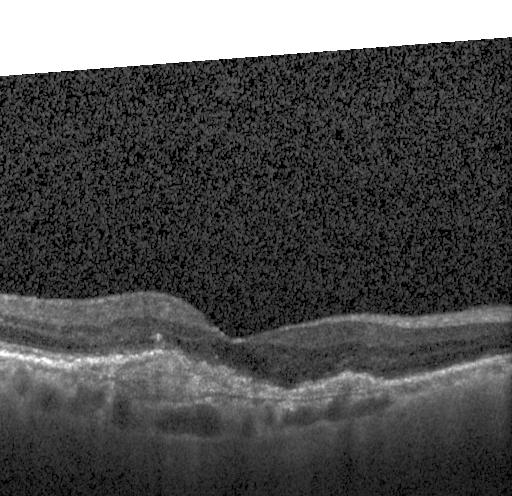

OCT B-scan; acquired on a Heidelberg Spectralis; horizontal scan through the fovea; spectral-domain OCT.
The scan shows CNV.